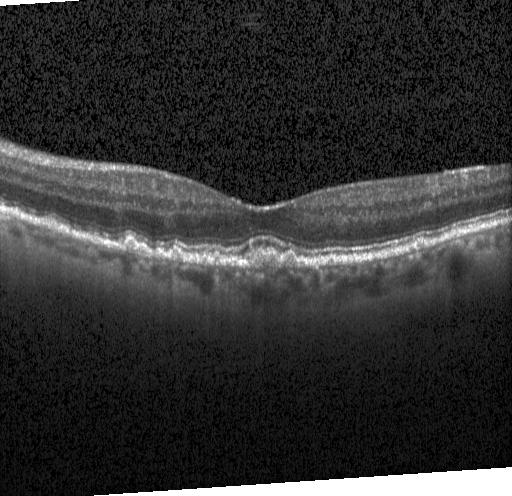 Spectral-domain optical coherence tomography · fovea-centered · optical coherence tomography B-scan
Finding: multiple drusen.